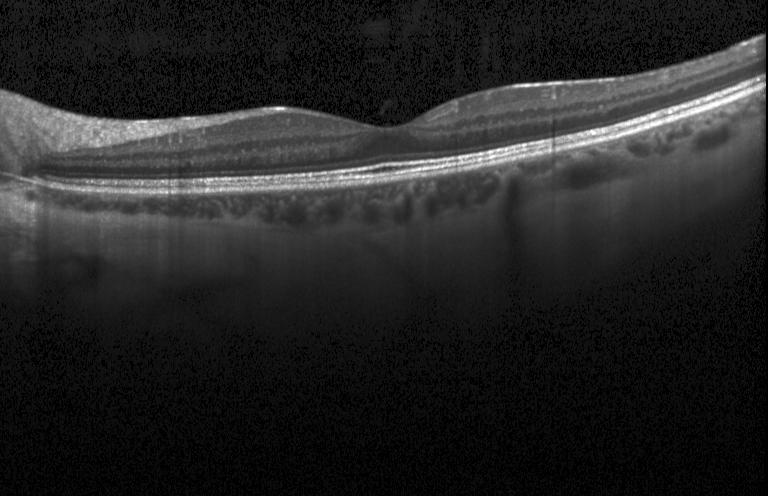
Optical coherence tomography scan — Impression: no evidence of CNV, DME, or drusen.